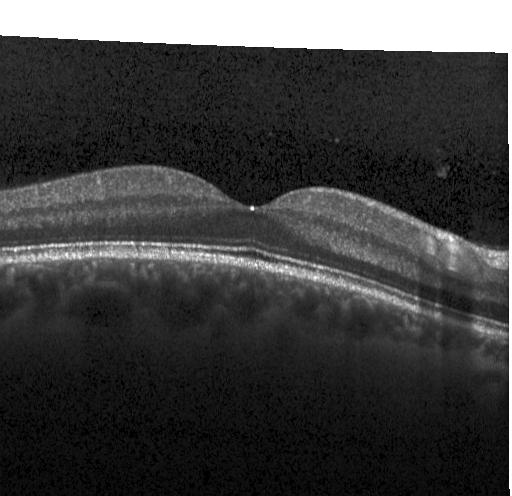
Spectral-domain OCT, retinal OCT B-scan.
Finding: neither choroidal neovascularization, diabetic macular edema, nor drusen.